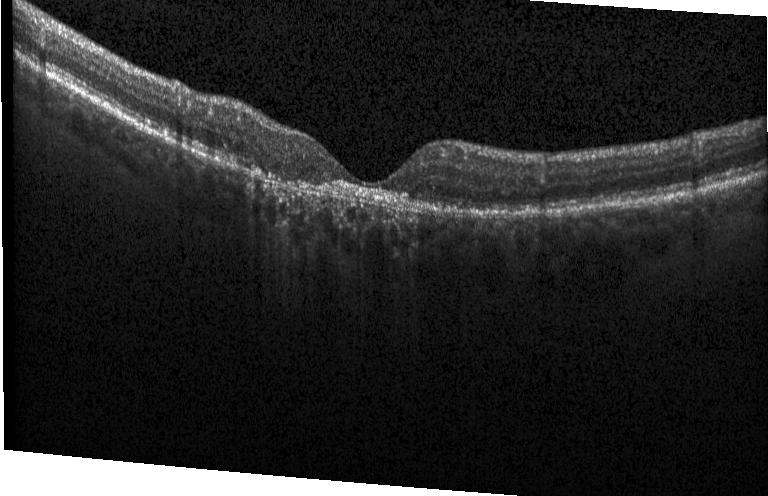
Macular OCT: a choroidal neovascular membrane.